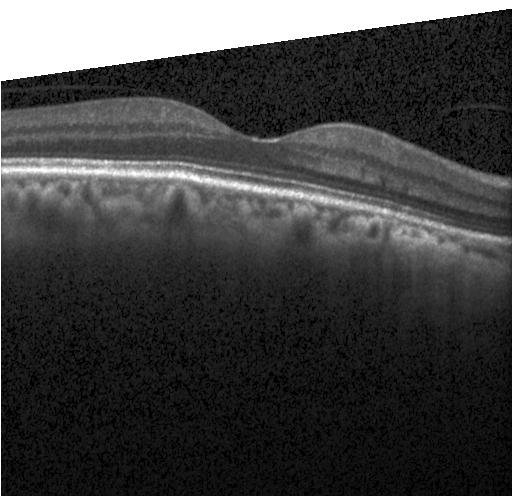

Assessment: no choroidal neovascularization, no diabetic macular edema, and no drusen.